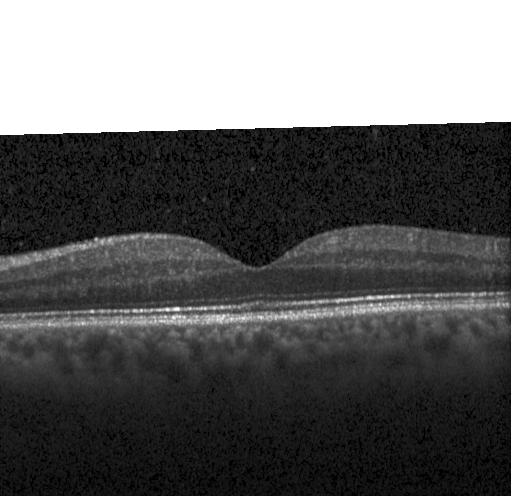

Dx: no CNV, DME, or drusen.